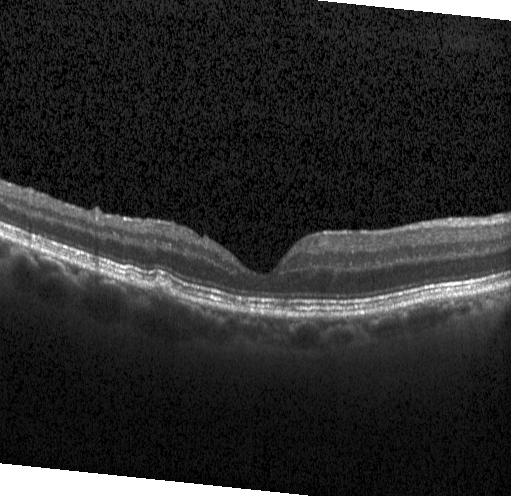 Optical coherence tomography B-scan. Dx: sub-RPE drusenoid deposits.